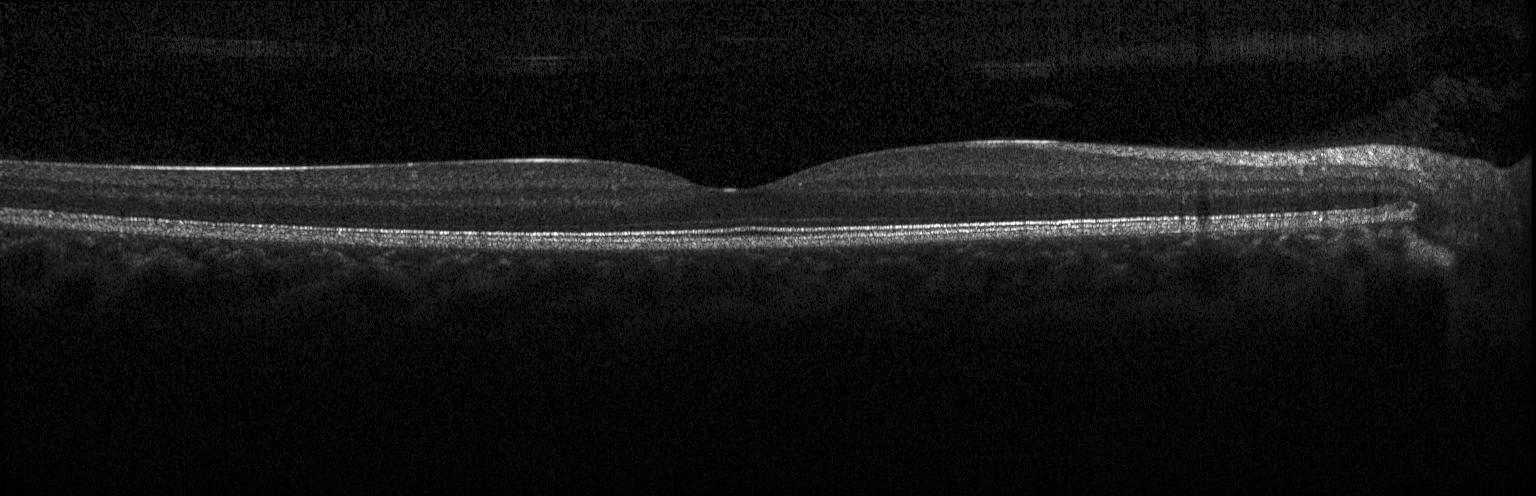

Optical coherence tomography scan; acquired on a Heidelberg Spectralis; SD-OCT; horizontal scan through the fovea.
This B-scan demonstrates no CNV, no DME, and no drusen.